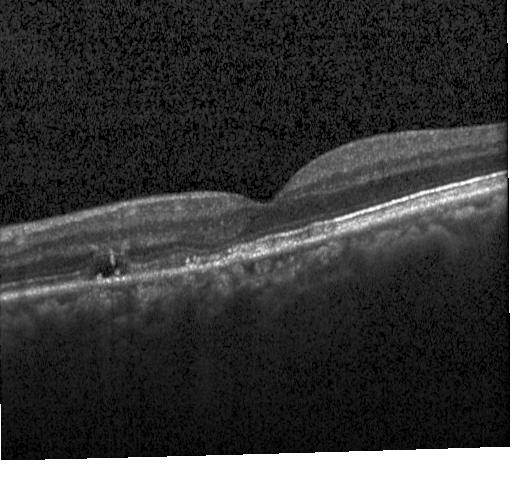 Spectral-domain optical coherence tomography · acquired on a Heidelberg Spectralis · retinal OCT B-scan · horizontal scan through the fovea.
Macular OCT: choroidal neovascularization (CNV).